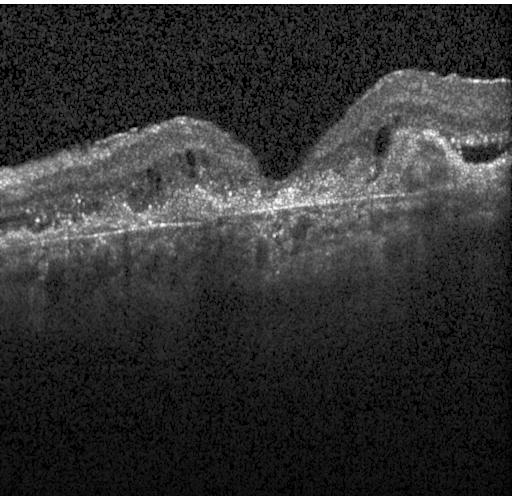 Finding: a choroidal neovascular membrane.